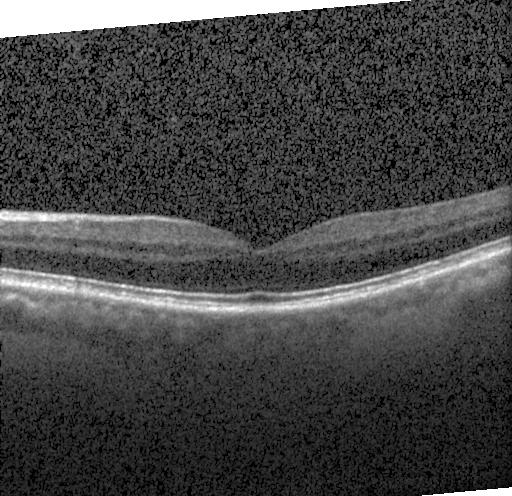 Retinal OCT B-scan. Heidelberg Spectralis OCT system. Through the macula. Spectral-domain OCT — No evidence of choroidal neovascularization, diabetic macular edema, or drusen.